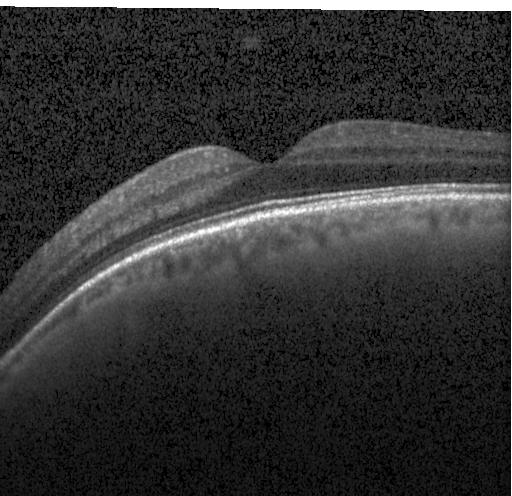
OCT B-scan — This B-scan demonstrates neither CNV, DME, nor drusen.